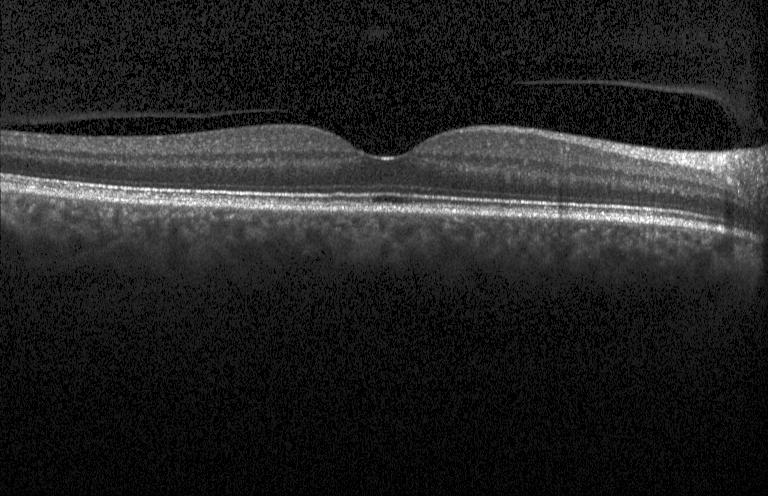

Diagnosis: no evidence of CNV, DME, or drusen.